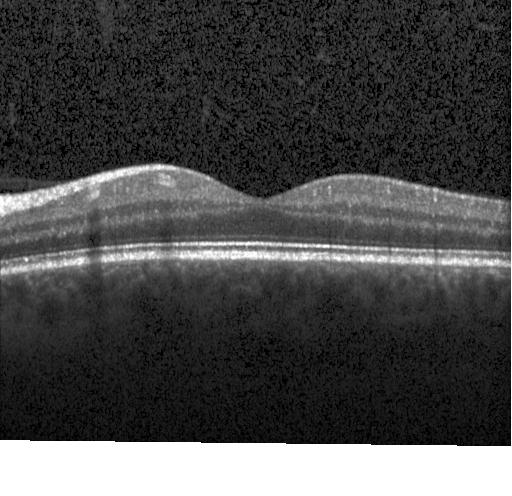

Diagnosis: no choroidal neovascularization, diabetic macular edema, or drusen.